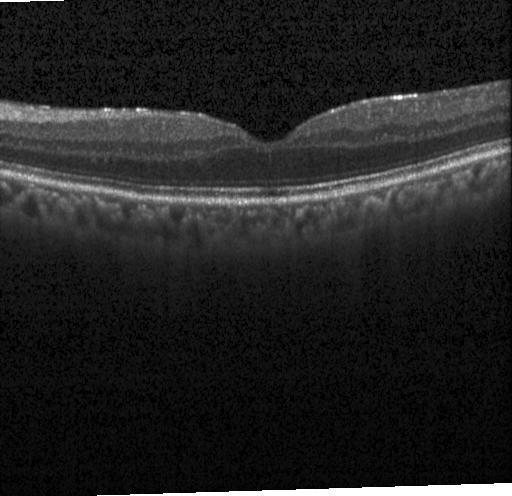 OCT B-scan showing no choroidal neovascularization, no diabetic macular edema, and no drusen.